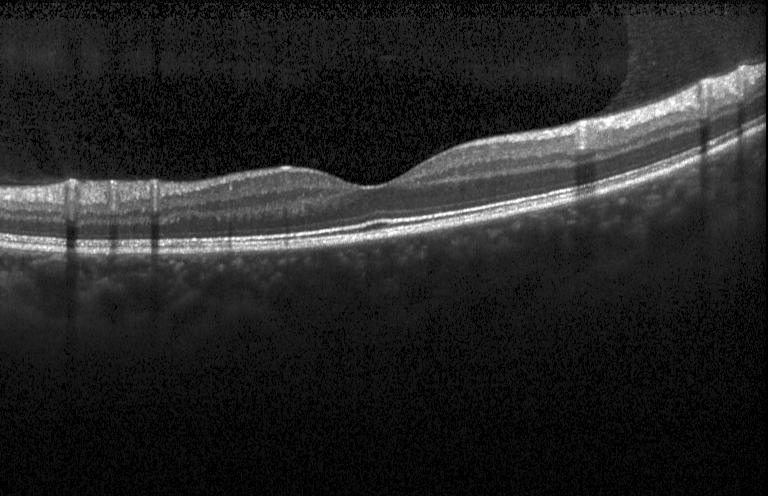
Diagnosis: no CNV, no DME, and no drusen.